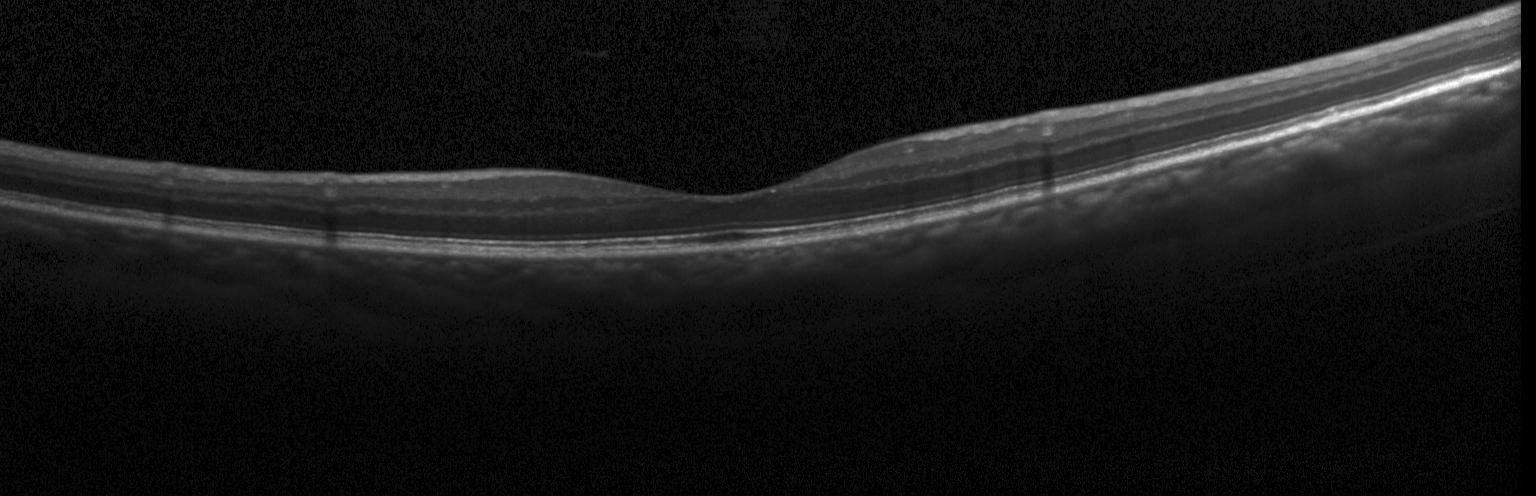

Finding: no choroidal neovascularization, no diabetic macular edema, and no drusen.